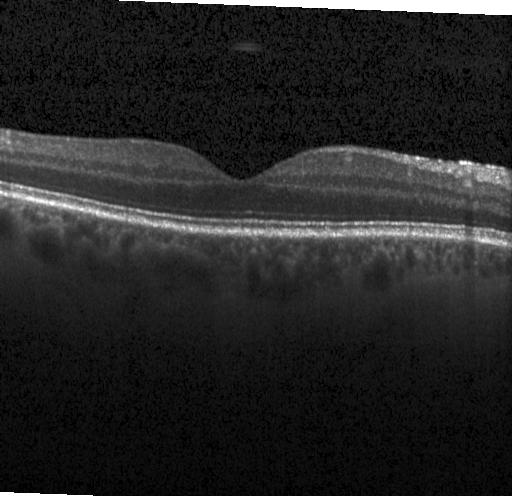

Instrument: Heidelberg Spectralis, fovea-centered, OCT B-scan, SD-OCT. Assessment: neither choroidal neovascularization, diabetic macular edema, nor drusen.